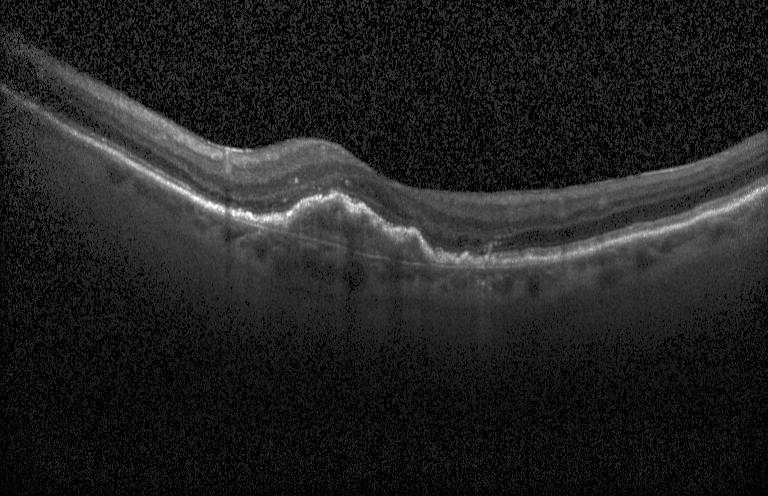
Spectral-domain OCT B-scan: choroidal neovascularization.